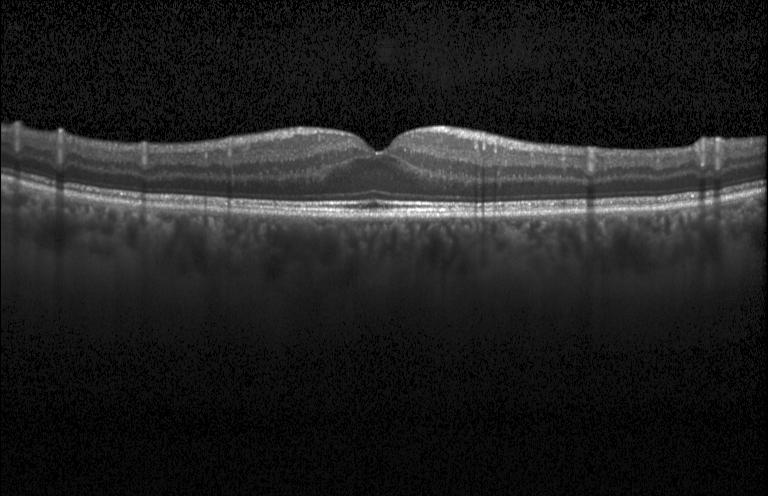
The scan shows no choroidal neovascularization, diabetic macular edema, or drusen.